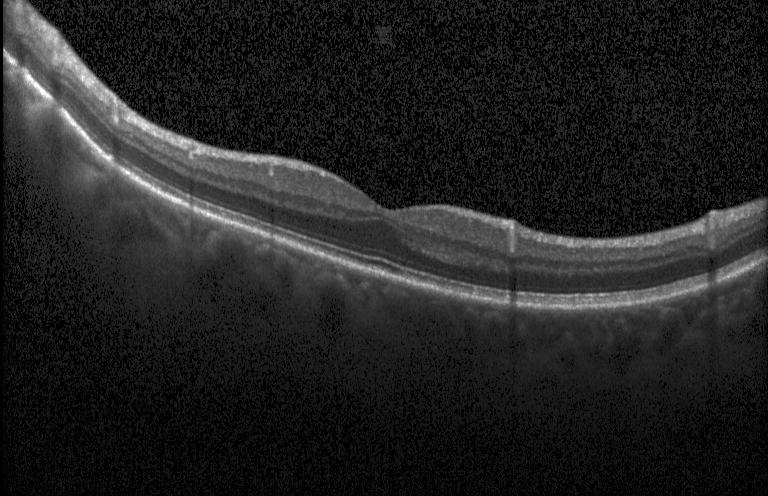
OCT B-scan
Diagnosis: neither CNV, DME, nor drusen.